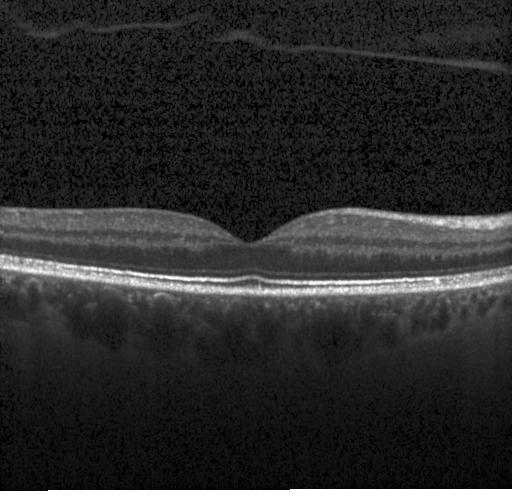
Retinal OCT B-scan · acquired on a Heidelberg Spectralis — OCT finding: no choroidal neovascularization, no diabetic macular edema, and no drusen.